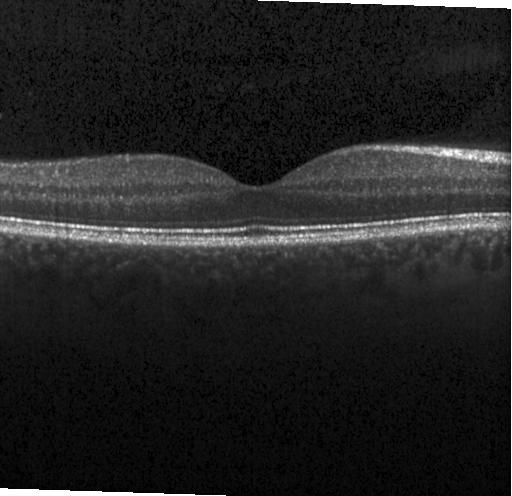 OCT finding: no choroidal neovascularization, diabetic macular edema, or drusen.